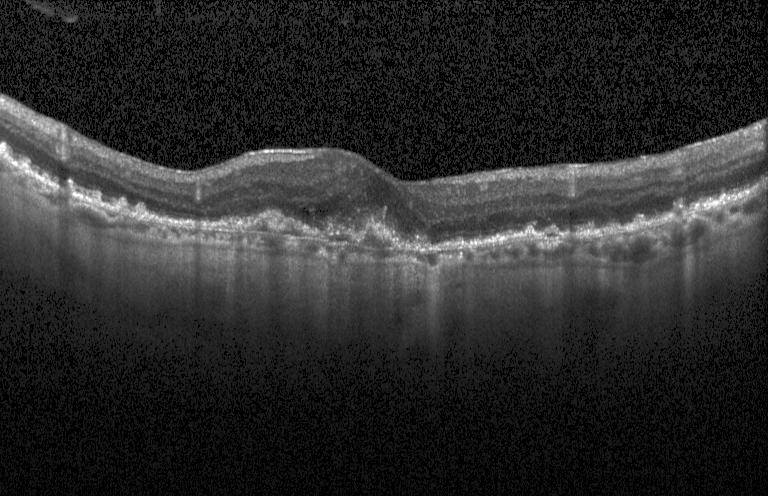
Impression: CNV.